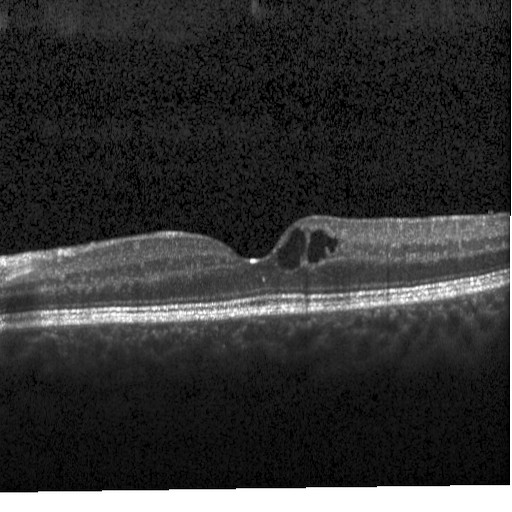

Dx: diabetic macular edema (DME).